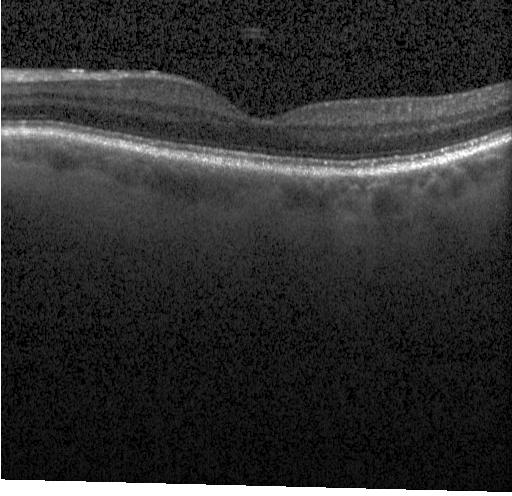
Optical coherence tomography scan; Heidelberg Spectralis — Finding: no choroidal neovascularization, diabetic macular edema, or drusen.